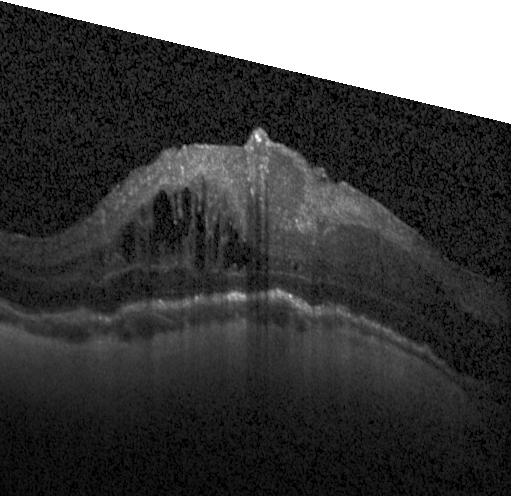

Retinal OCT B-scan; horizontal scan through the fovea
Diagnosis: diabetic macular edema (DME).